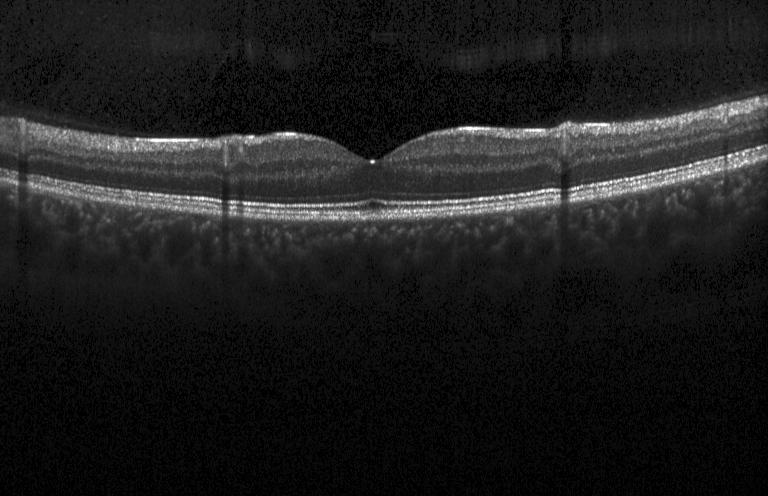 Retinal OCT B-scan
Finding: no choroidal neovascularization, diabetic macular edema, or drusen.